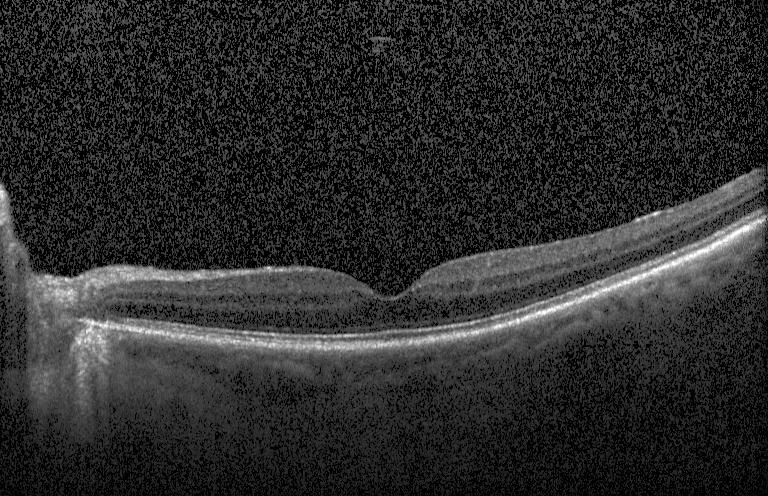

Macular OCT: no choroidal neovascularization, diabetic macular edema, or drusen.